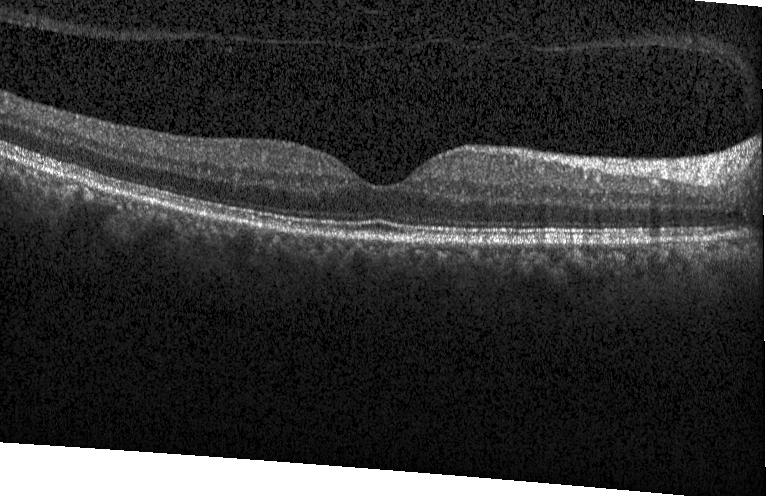 This B-scan demonstrates no choroidal neovascularization, no diabetic macular edema, and no drusen.